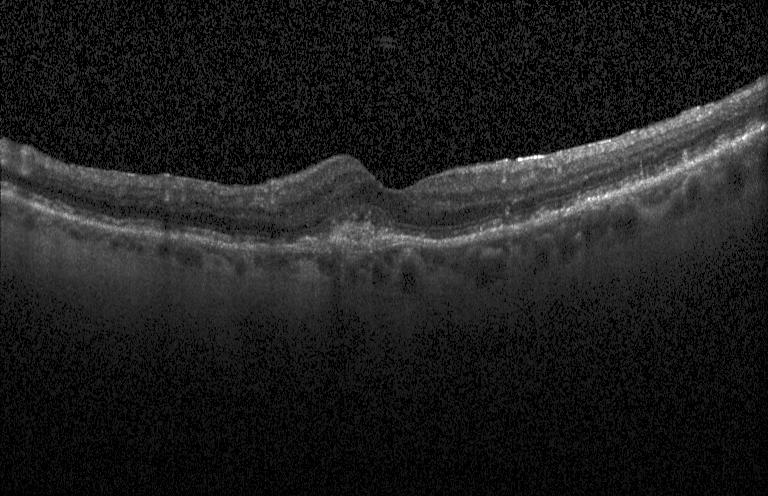
Finding: a choroidal neovascular membrane.